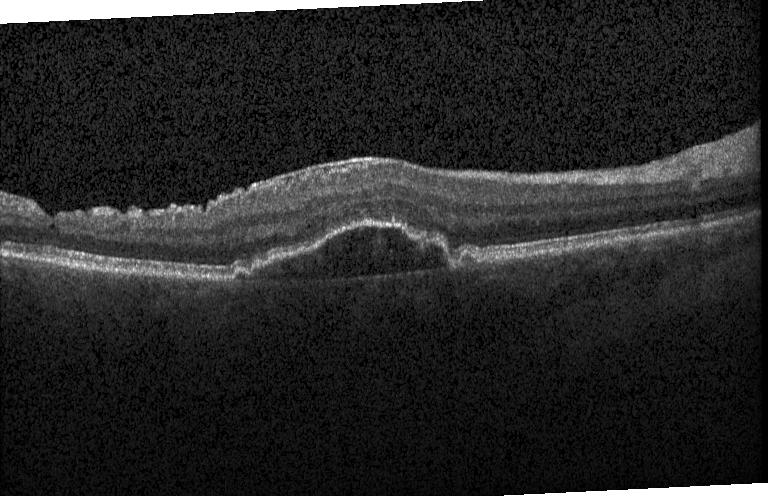 OCT finding: a choroidal neovascular membrane.